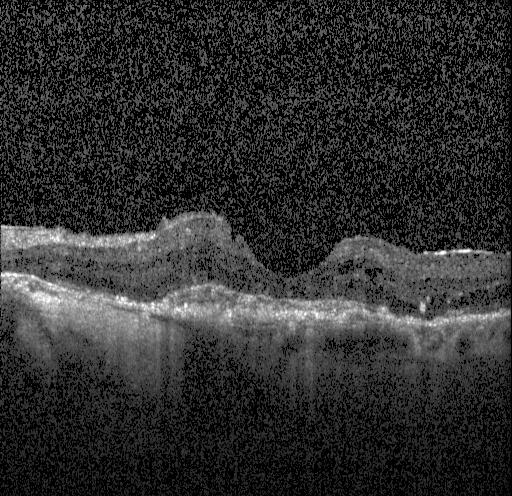 Optical coherence tomography B-scan, through the macula, Heidelberg Spectralis OCT system, SD-OCT. Macular OCT: a choroidal neovascular membrane.